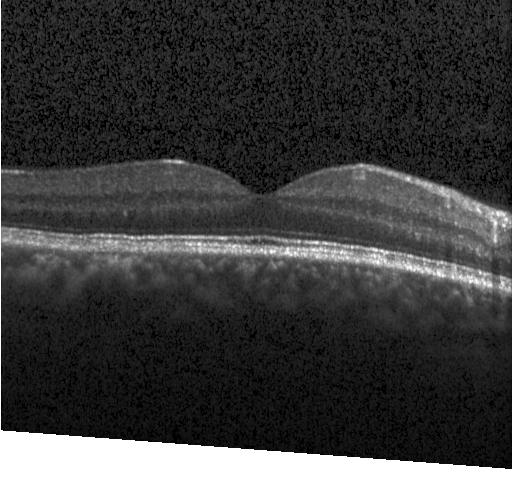

Optical coherence tomography scan, centered on the fovea, acquired on a Heidelberg Spectralis, SD-OCT. Dx: neither choroidal neovascularization, diabetic macular edema, nor drusen.